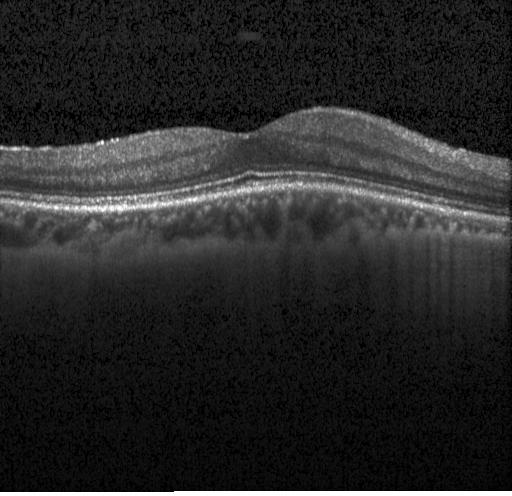 Macular OCT: no evidence of choroidal neovascularization, diabetic macular edema, or drusen.